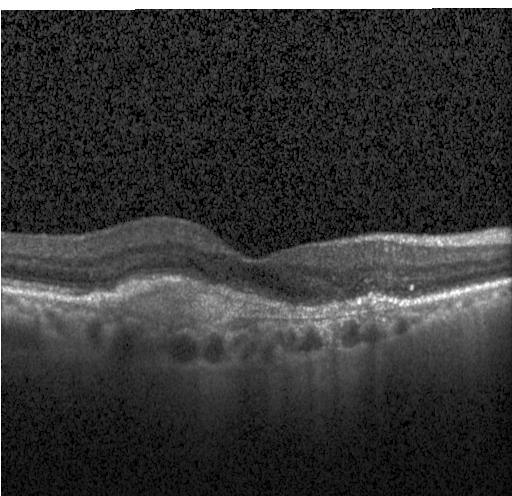
Spectral-domain OCT B-scan: choroidal neovascularization.